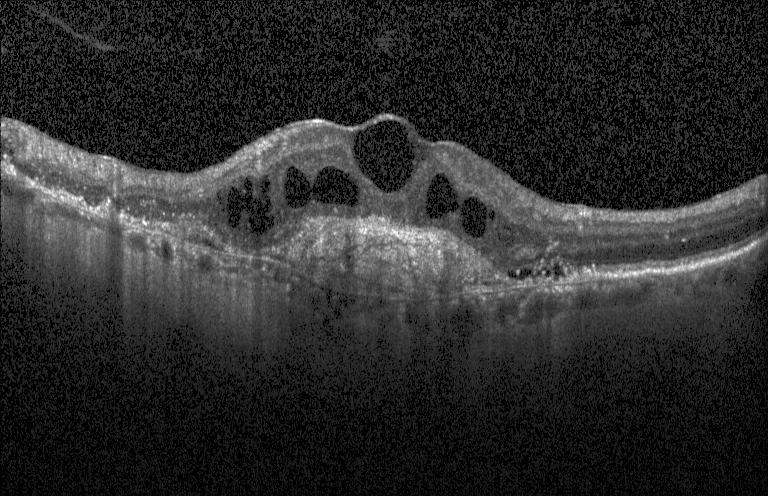 Diagnosis: choroidal neovascularization (CNV).